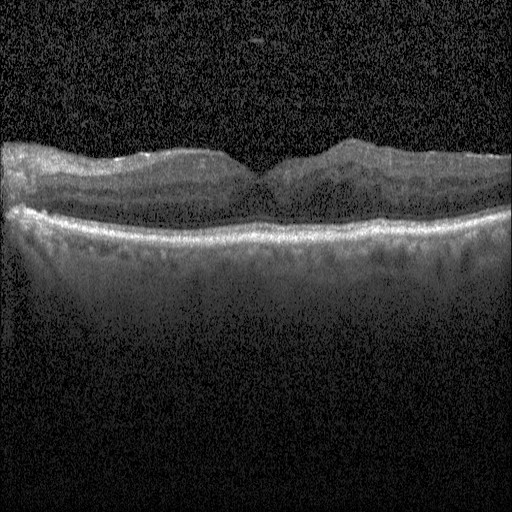 This B-scan demonstrates diabetic macular edema (DME).